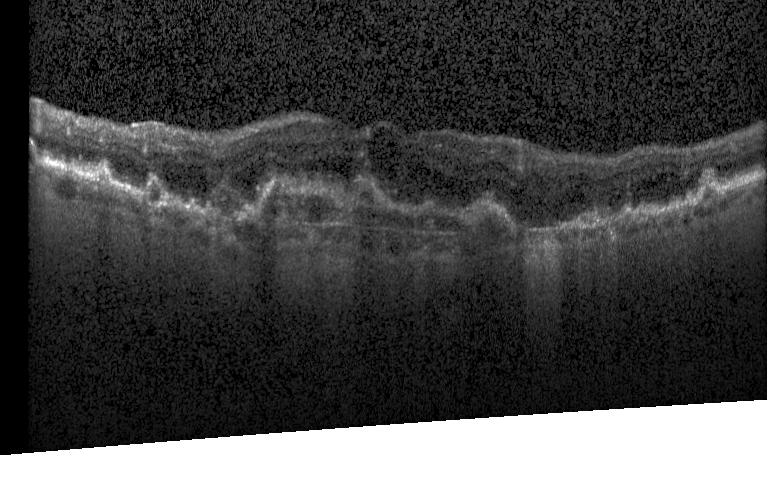
Horizontal scan through the fovea. Retinal OCT B-scan. SD-OCT. Acquired on a Heidelberg Spectralis
Impression: a choroidal neovascular membrane.